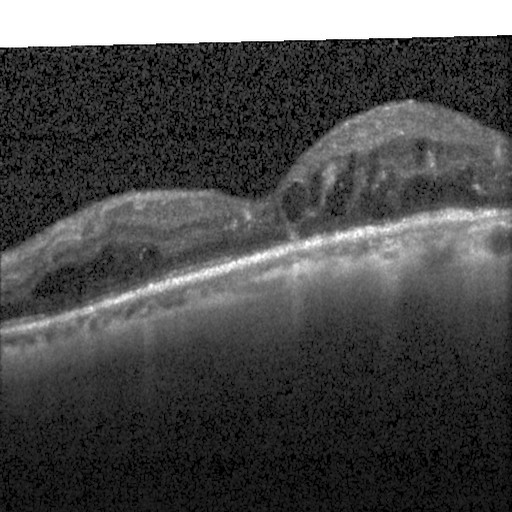 Finding: DME.